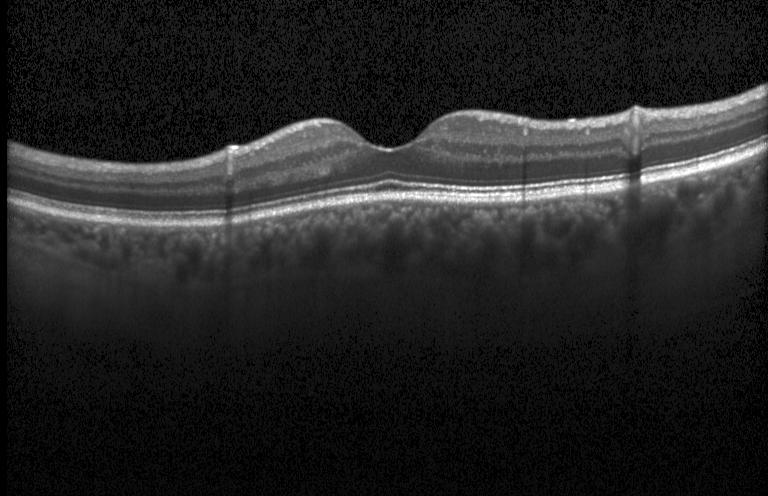

Optical coherence tomography scan. Horizontal scan through the fovea — Macular OCT: no CNV, DME, or drusen.